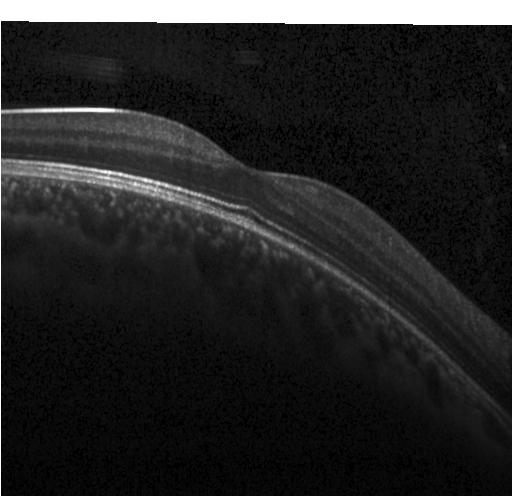 Diagnosis: no evidence of CNV, DME, or drusen.